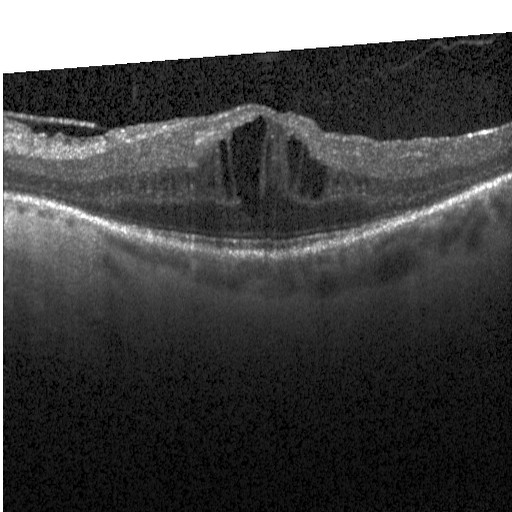
OCT line scan · Heidelberg Spectralis OCT system · spectral-domain OCT. Diagnosis: DME.